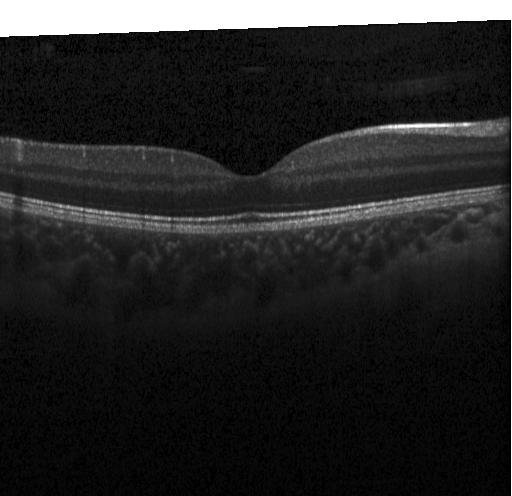
Spectral-domain OCT · Heidelberg Spectralis OCT system · through the macula · optical coherence tomography scan — Diagnosis: no CNV, no DME, and no drusen.